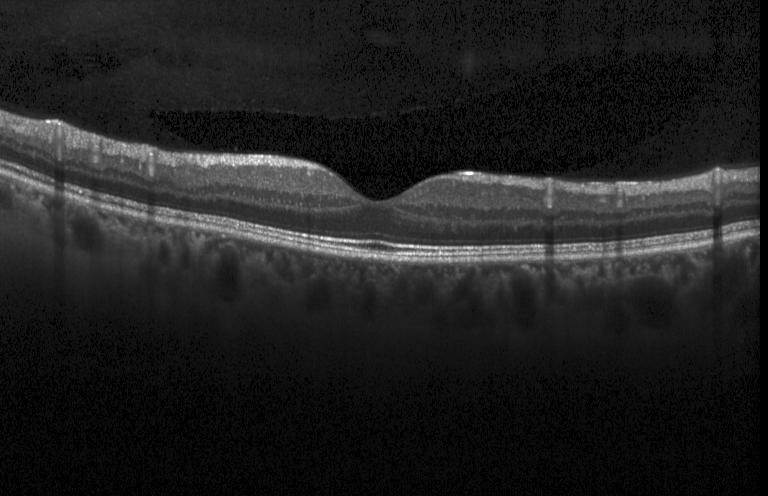

Diagnosis: no evidence of choroidal neovascularization, diabetic macular edema, or drusen.